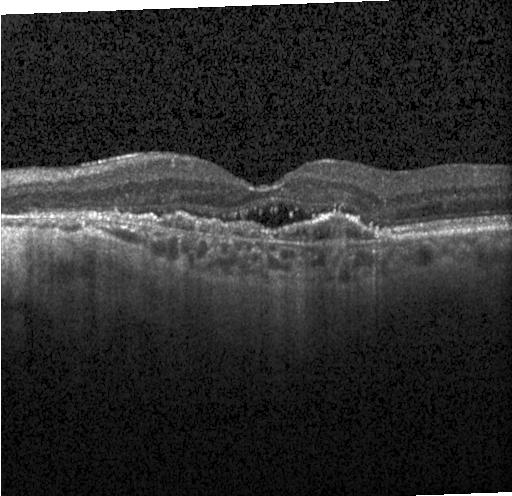

Spectral-domain OCT B-scan: choroidal neovascularization.